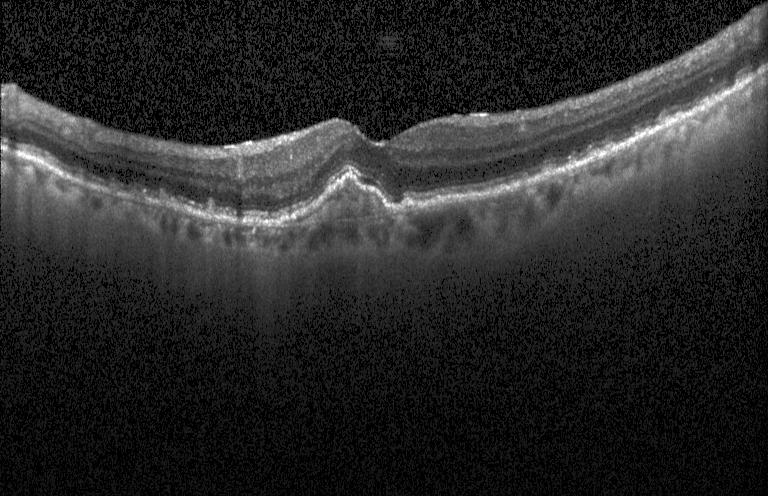 Dx: a choroidal neovascular membrane.